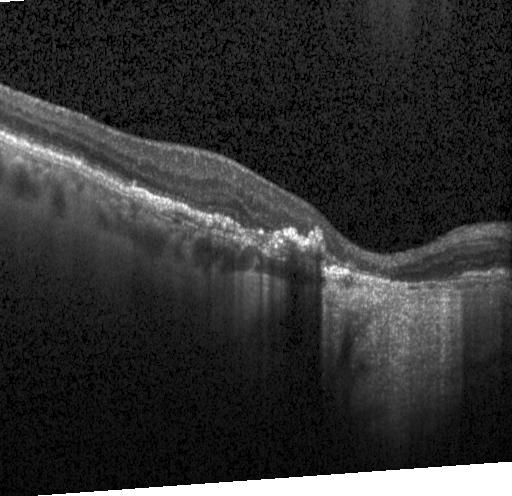
Acquired on a Heidelberg Spectralis · optical coherence tomography scan
Assessment: a choroidal neovascular membrane.